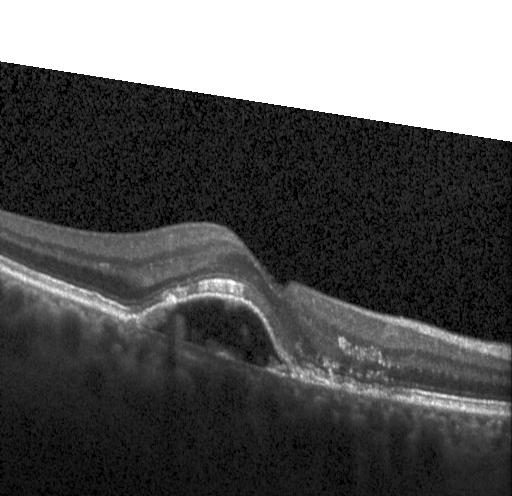
Centered on the fovea. Instrument: Heidelberg Spectralis. Retinal OCT cross-section. Diagnosis: a choroidal neovascular membrane.